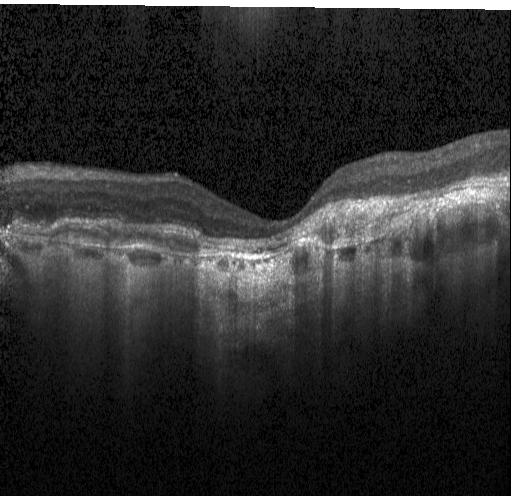 Optical coherence tomography scan. Diagnosis: a choroidal neovascular membrane.